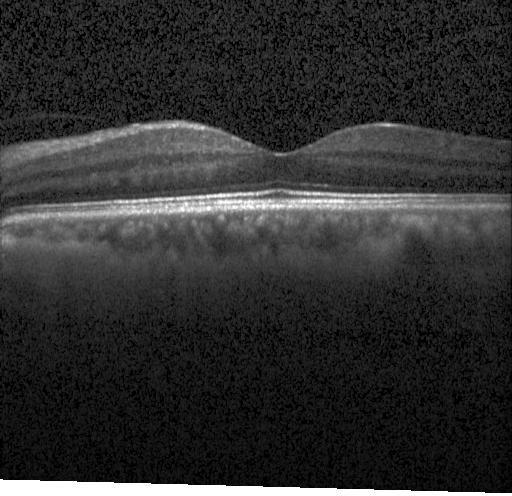

Dx: no evidence of choroidal neovascularization, diabetic macular edema, or drusen.